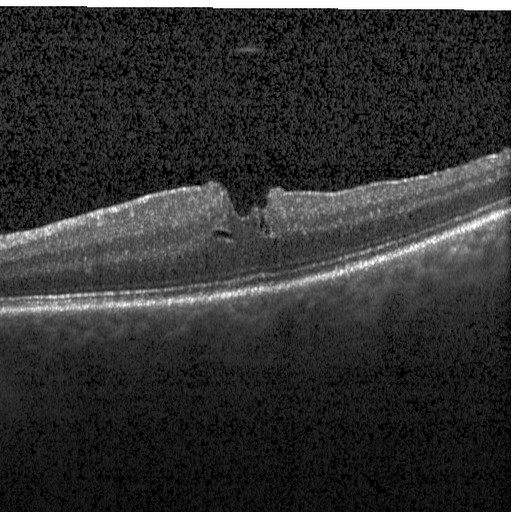
DME.